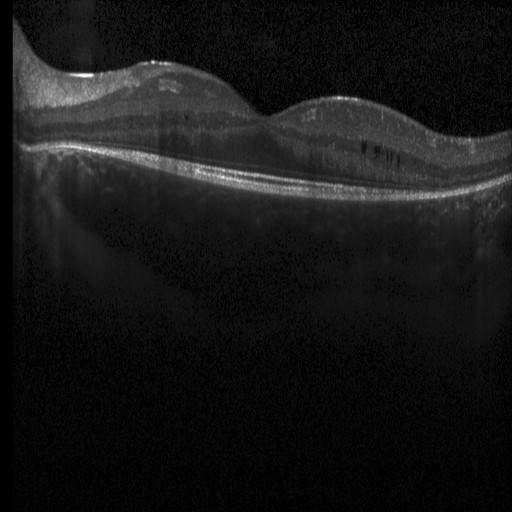 OCT B-scan — Finding: DME.